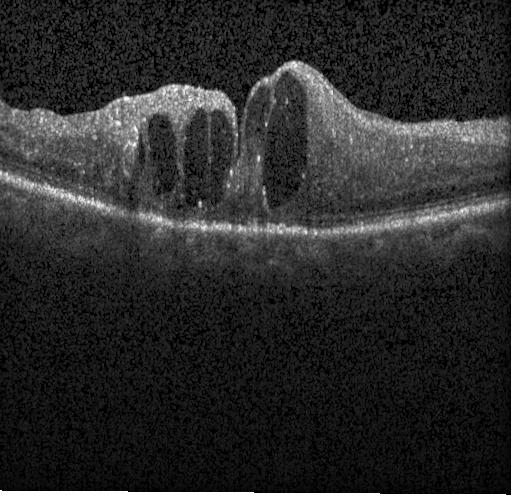
OCT line scan, Heidelberg Spectralis OCT system
DME.